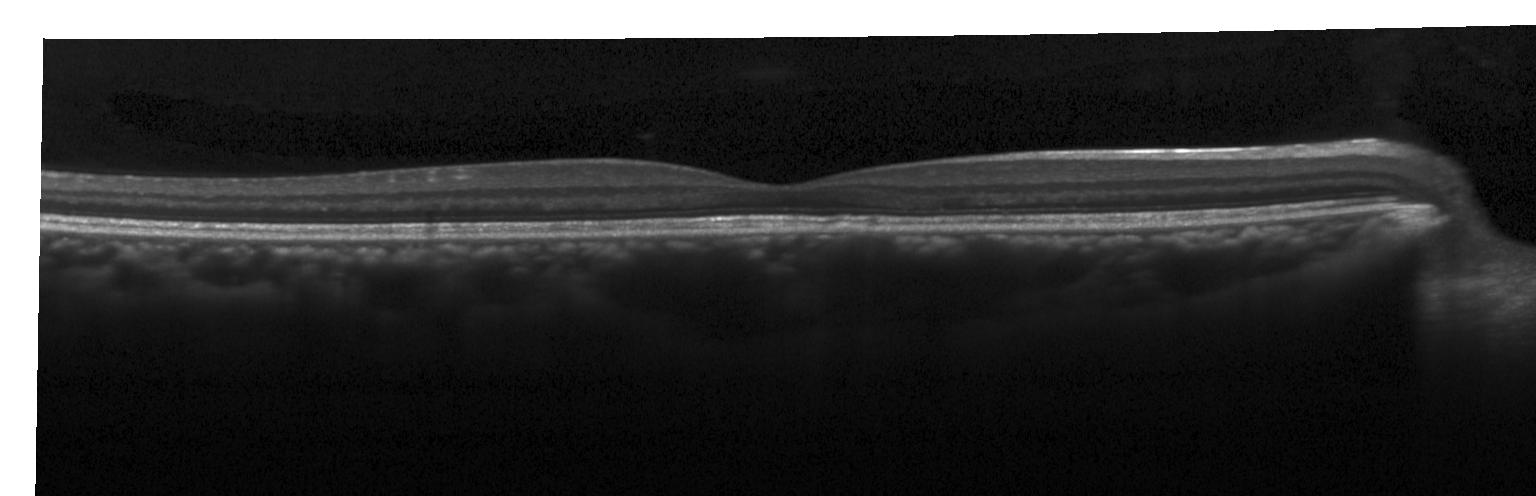

Diagnosis: neither choroidal neovascularization, diabetic macular edema, nor drusen.